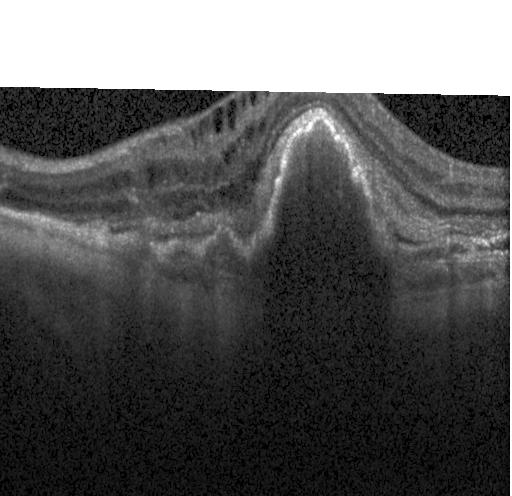

OCT finding: a choroidal neovascular membrane.